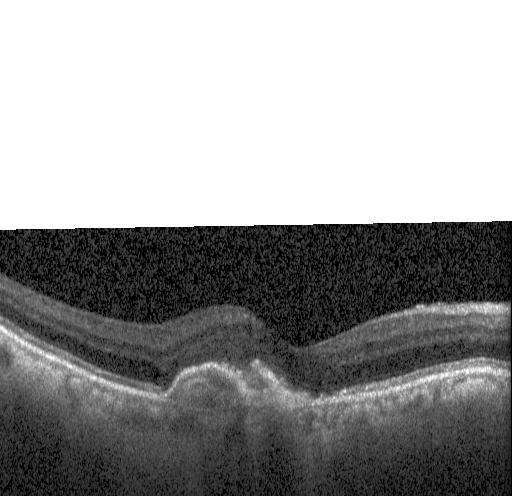

Through the macula; SD-OCT; OCT line scan.
Choroidal neovascularization (CNV).